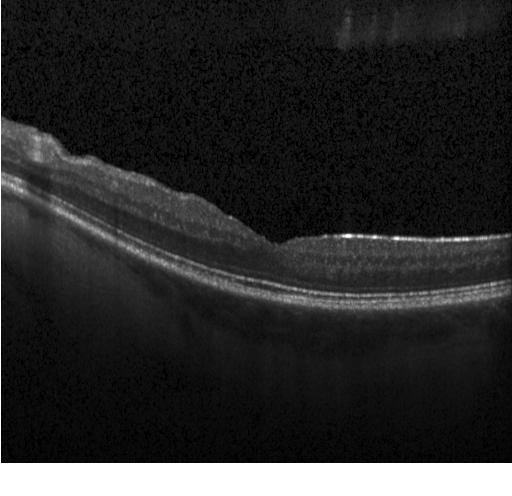
OCT line scan, spectral-domain OCT — Macular OCT: no CNV, no DME, and no drusen.